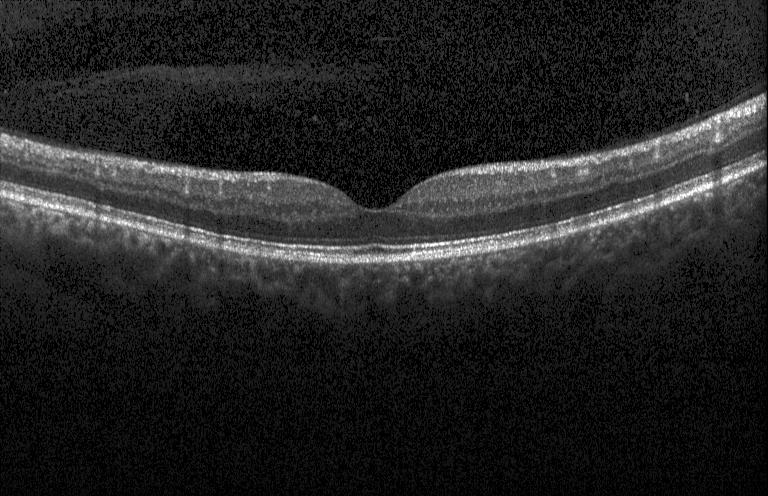 Retinal OCT B-scan.
Diagnosis: no choroidal neovascularization, no diabetic macular edema, and no drusen.